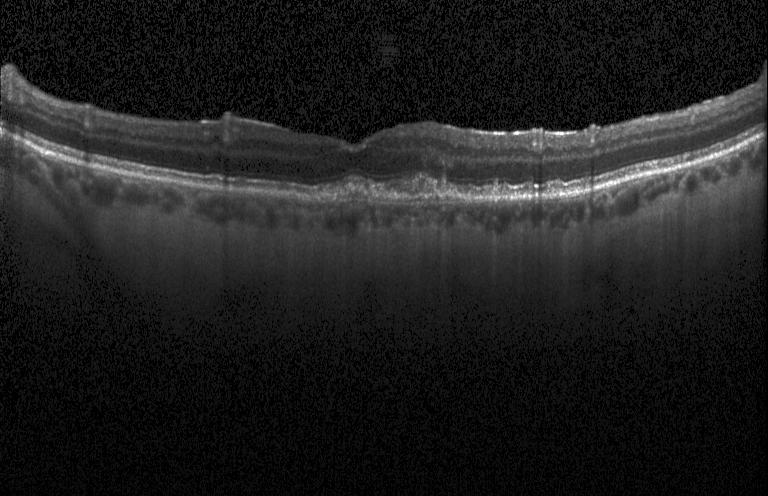
Spectral-domain OCT, OCT line scan, horizontal scan through the fovea
OCT finding: multiple drusen.